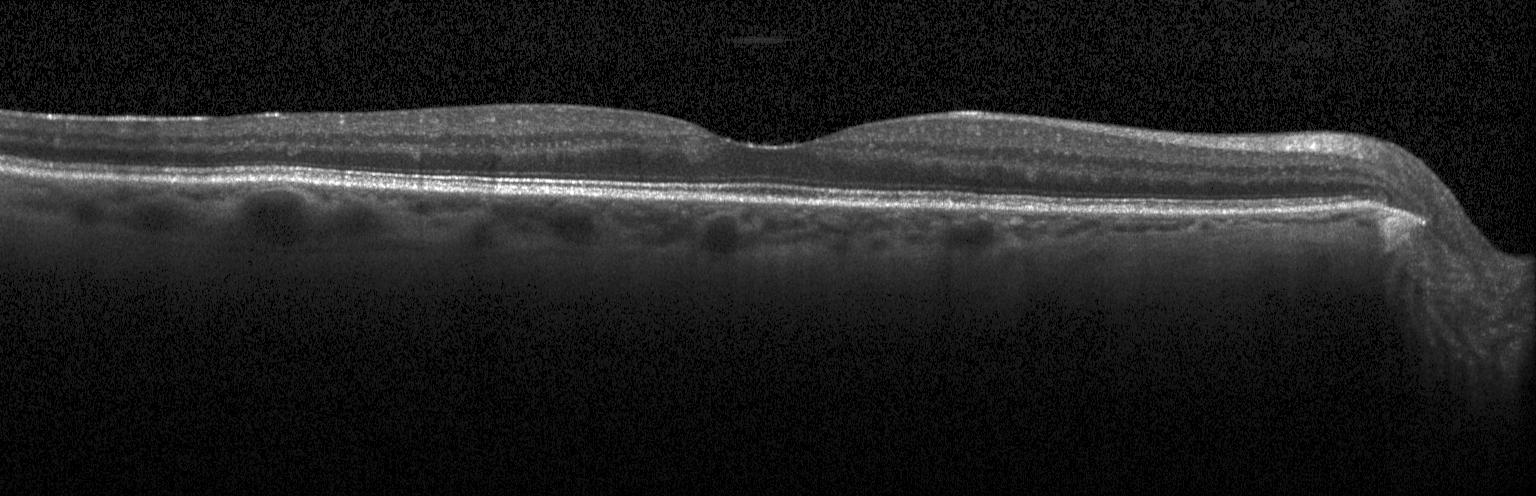
OCT B-scan · spectral-domain optical coherence tomography · instrument: Heidelberg Spectralis.
Impression: neither choroidal neovascularization, diabetic macular edema, nor drusen.